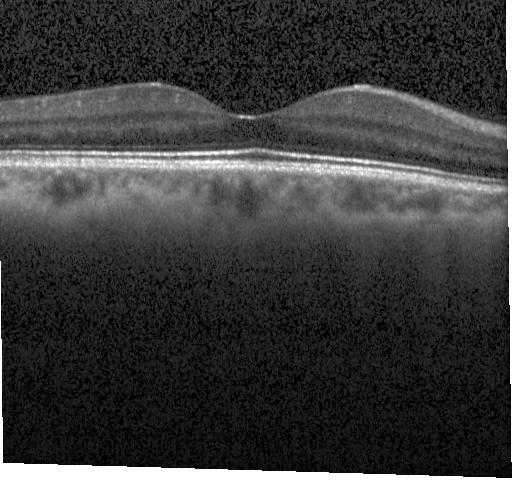 OCT line scan, spectral-domain OCT. Impression: no choroidal neovascularization, diabetic macular edema, or drusen.